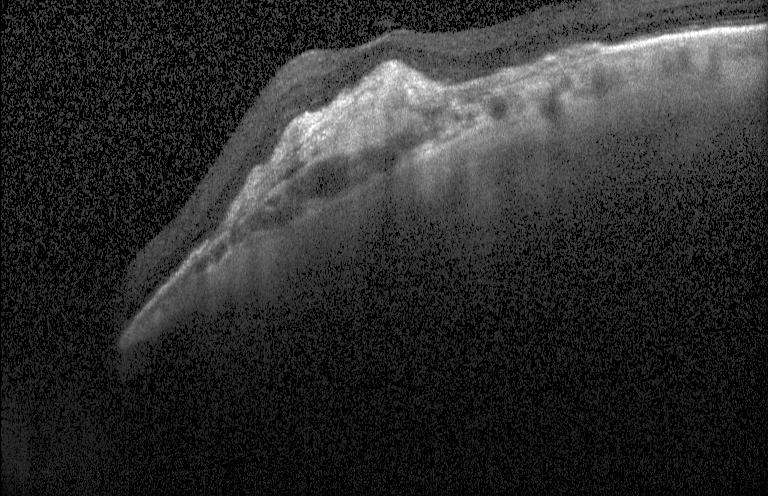
Impression: CNV.